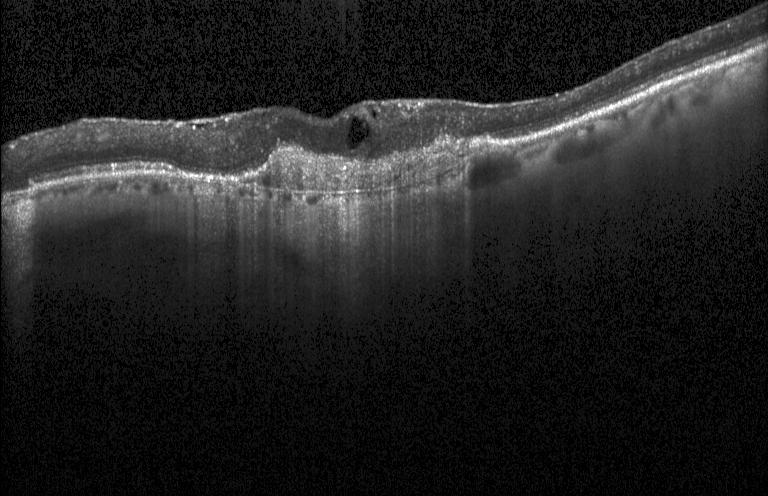
Heidelberg Spectralis OCT system, OCT B-scan, centered on the fovea, spectral-domain optical coherence tomography
Dx: a choroidal neovascular membrane.